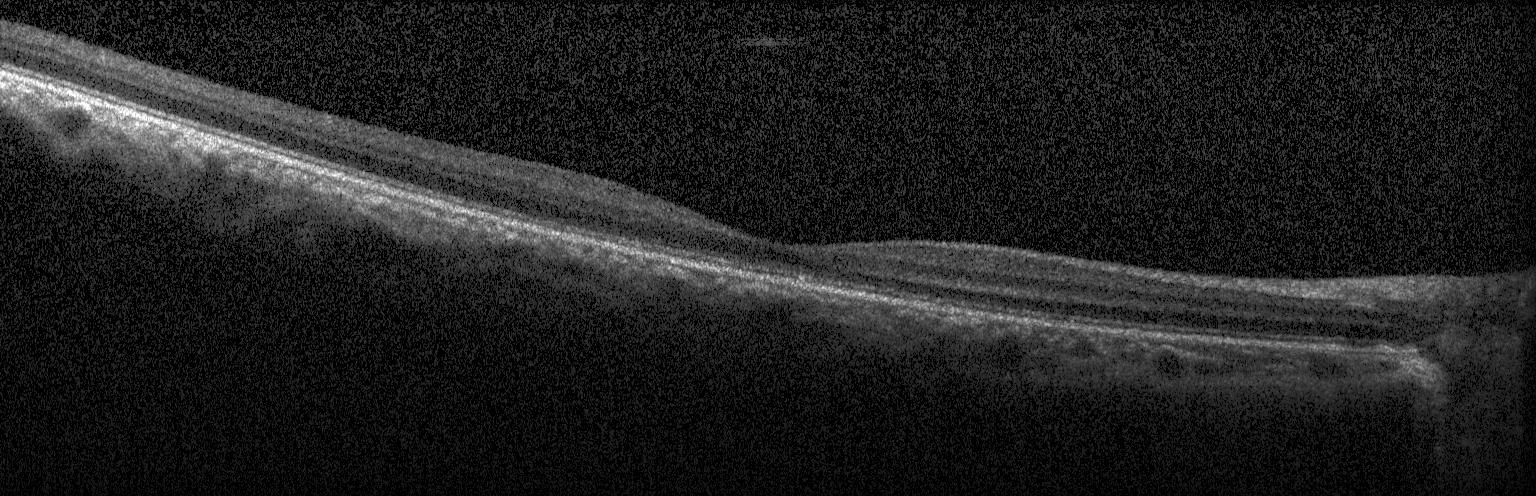
Acquired on a Heidelberg Spectralis. Centered on the fovea. Optical coherence tomography B-scan.
No evidence of choroidal neovascularization, diabetic macular edema, or drusen.